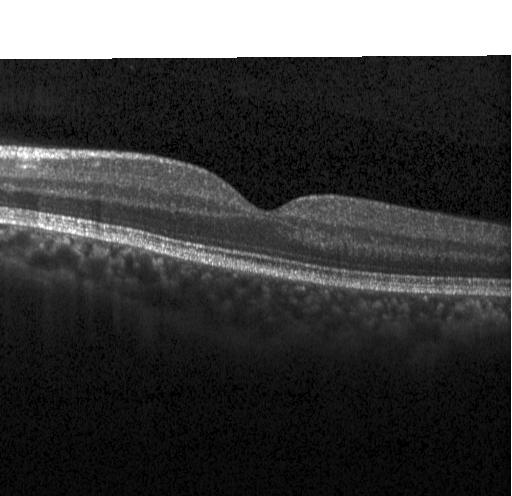 Optical coherence tomography B-scan.
OCT finding: no choroidal neovascularization, no diabetic macular edema, and no drusen.